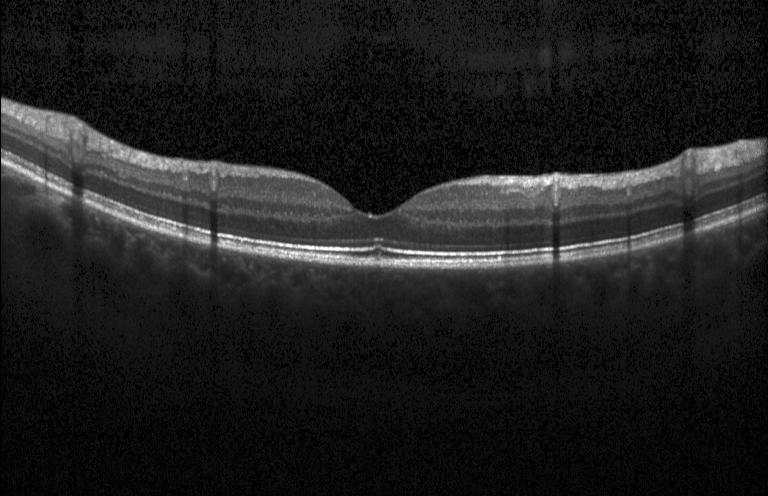

Retinal OCT cross-section. Instrument: Heidelberg Spectralis.
Diagnosis: neither choroidal neovascularization, diabetic macular edema, nor drusen.